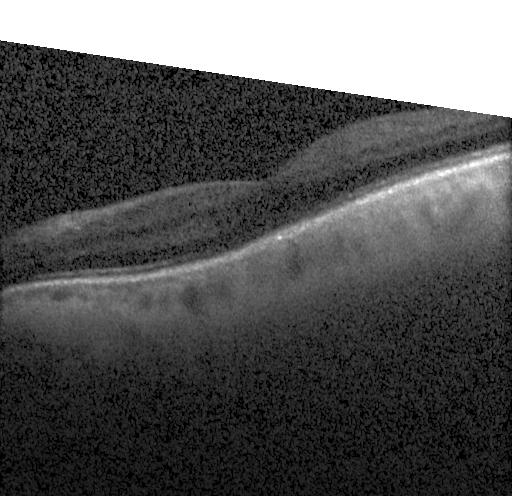

Diagnosis: no CNV, DME, or drusen.